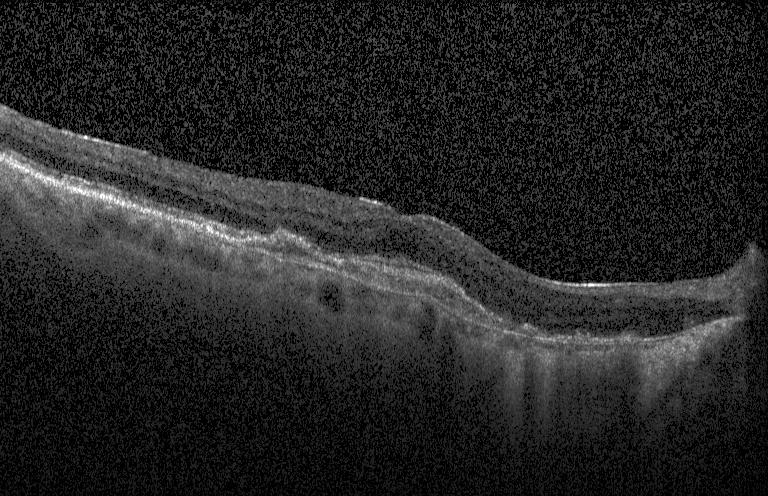 Retinal OCT B-scan · Heidelberg Spectralis · spectral-domain OCT
This B-scan demonstrates a choroidal neovascular membrane.